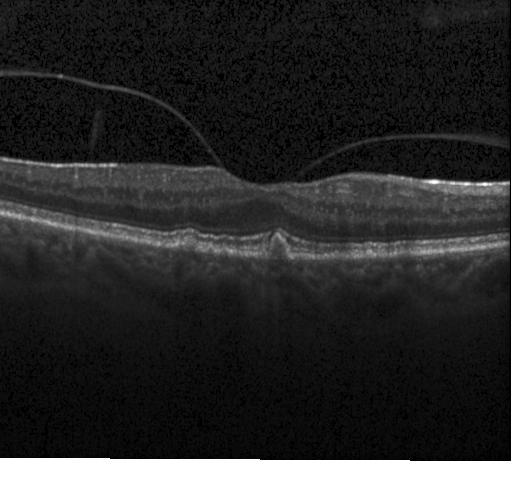

Impression: multiple drusen.